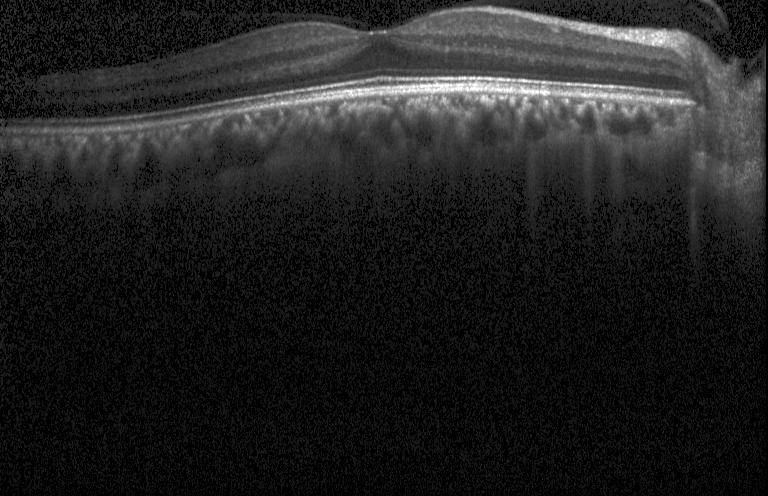 Optical coherence tomography B-scan.
Macular OCT: no evidence of choroidal neovascularization, diabetic macular edema, or drusen.